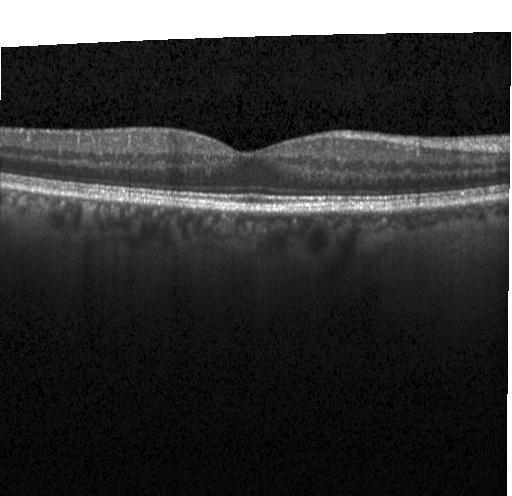 Spectral-domain OCT · through the macula · retinal OCT cross-section · Heidelberg Spectralis OCT system. No CNV, no DME, and no drusen.